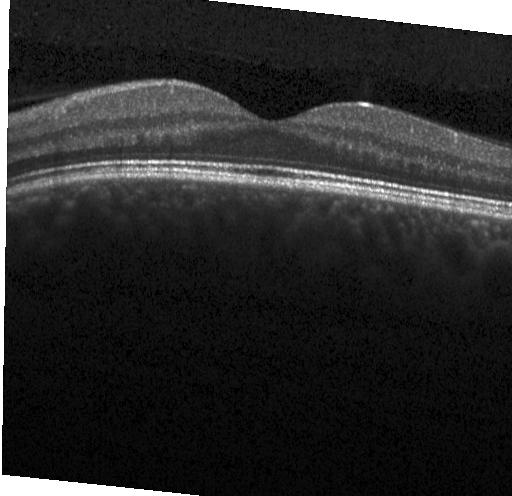

Macular OCT: no choroidal neovascularization, diabetic macular edema, or drusen.